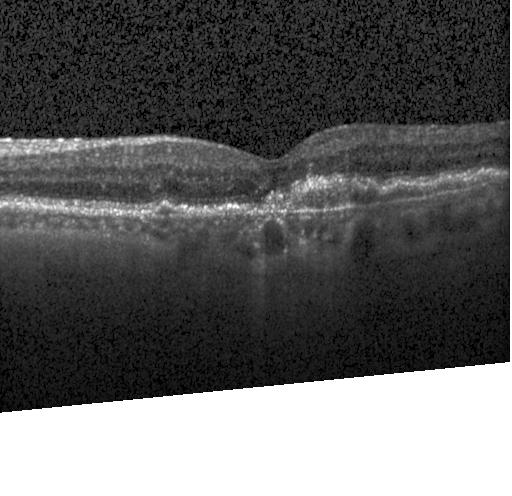

OCT line scan. Horizontal scan through the fovea. Dx: choroidal neovascularization (CNV).